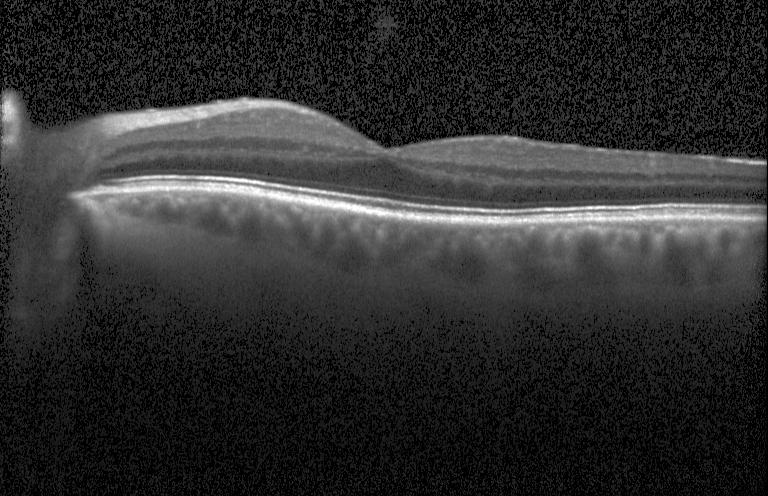

OCT finding: no evidence of choroidal neovascularization, diabetic macular edema, or drusen.